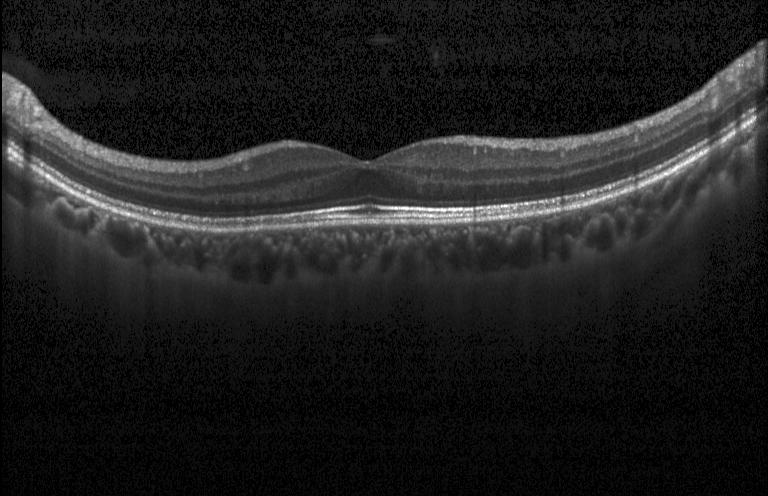

OCT B-scan
Finding: no choroidal neovascularization, diabetic macular edema, or drusen.